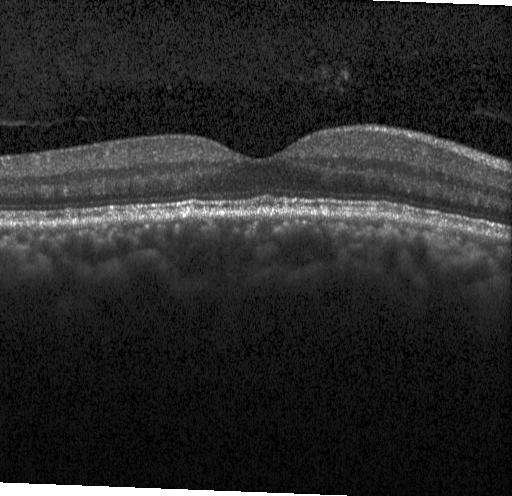
Macular OCT: drusen.